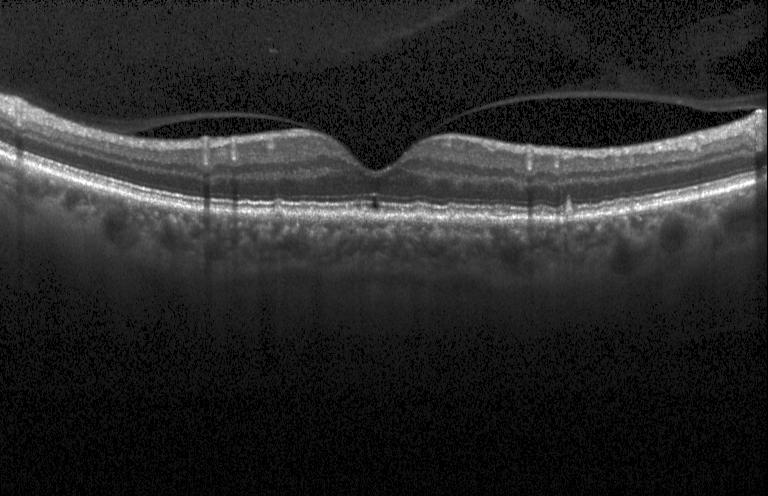

Finding: sub-RPE drusenoid deposits.